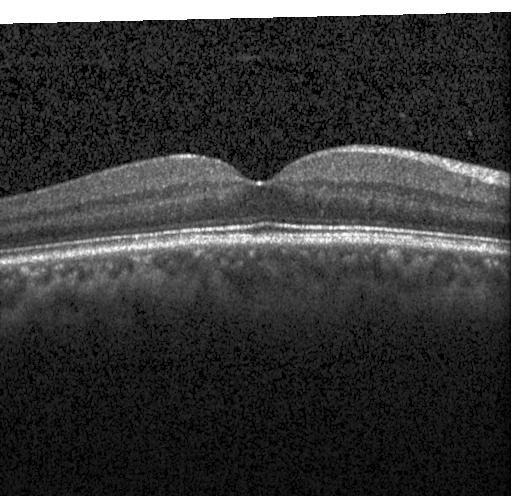

Retinal OCT B-scan · spectral-domain OCT
Impression: no choroidal neovascularization, diabetic macular edema, or drusen.